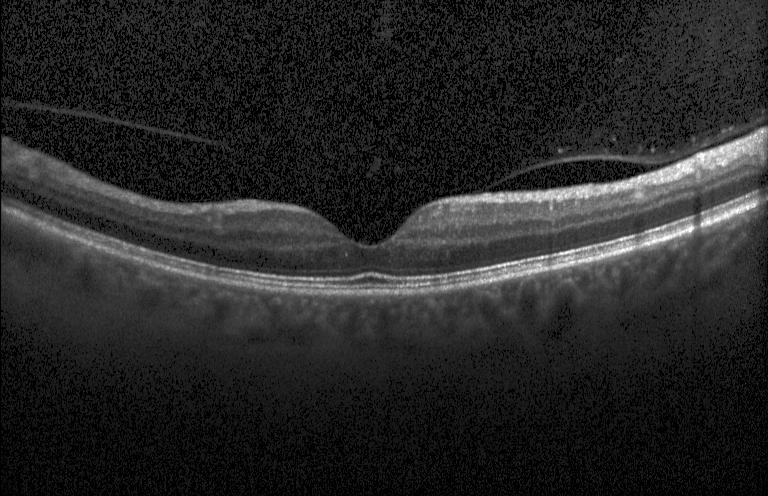

Spectral-domain optical coherence tomography · retinal OCT cross-section — The scan shows neither choroidal neovascularization, diabetic macular edema, nor drusen.